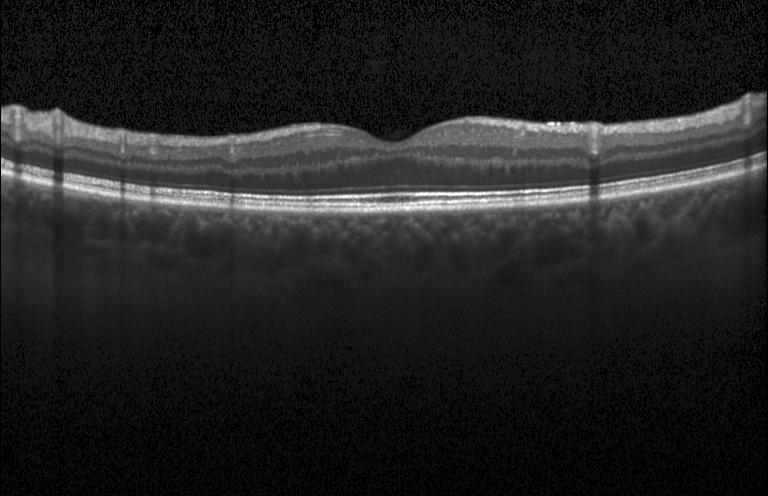

OCT B-scan.
Macular OCT: no choroidal neovascularization, diabetic macular edema, or drusen.